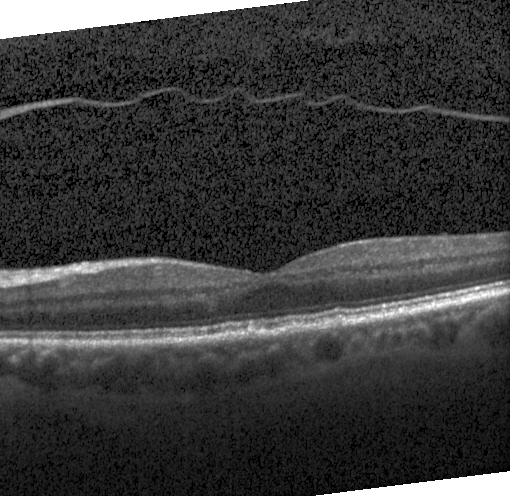 Optical coherence tomography B-scan.
Finding: multiple drusen.